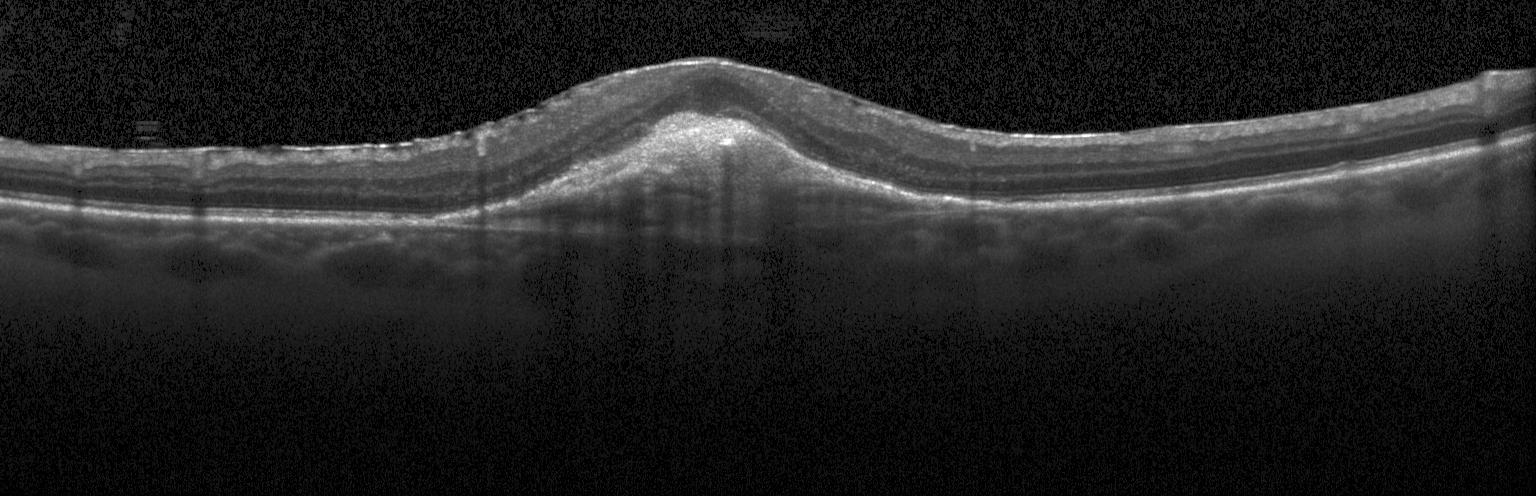
Macular OCT: a choroidal neovascular membrane.